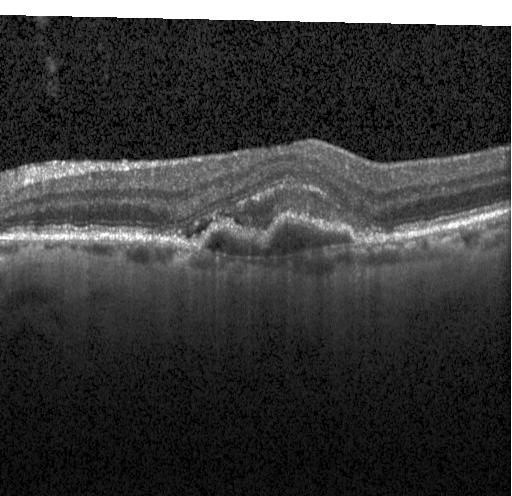

Retinal OCT B-scan; macular scan; instrument: Heidelberg Spectralis. Dx: choroidal neovascularization (CNV).